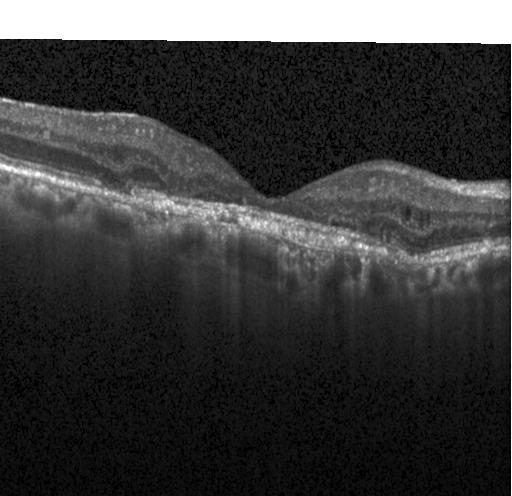 SD-OCT, retinal OCT B-scan, instrument: Heidelberg Spectralis.
Finding: CNV.